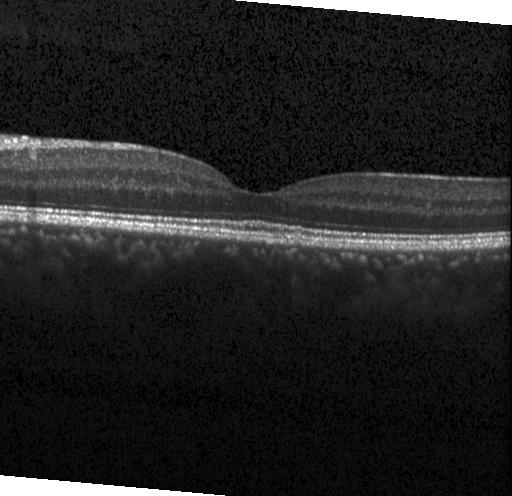
Retinal OCT B-scan.
Finding: no evidence of choroidal neovascularization, diabetic macular edema, or drusen.